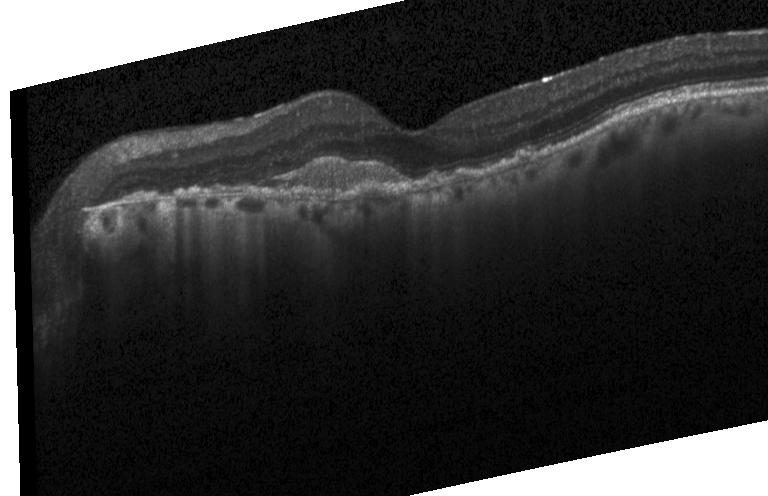

OCT B-scan showing a choroidal neovascular membrane.